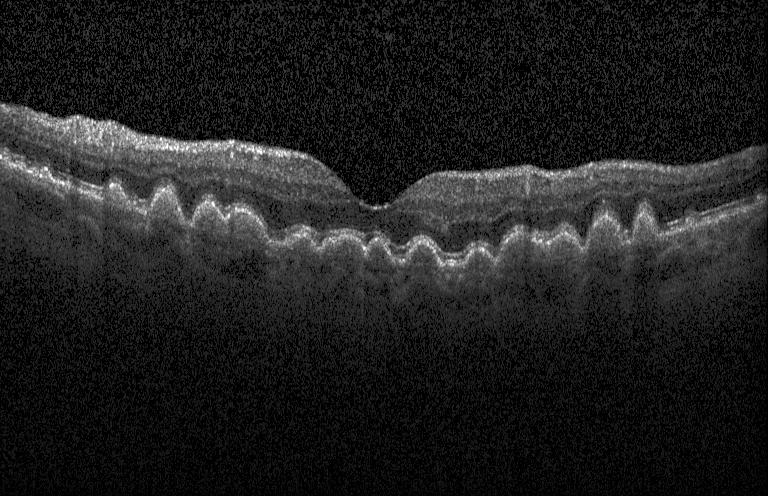
Optical coherence tomography scan. Fovea-centered
Dx: multiple drusen.